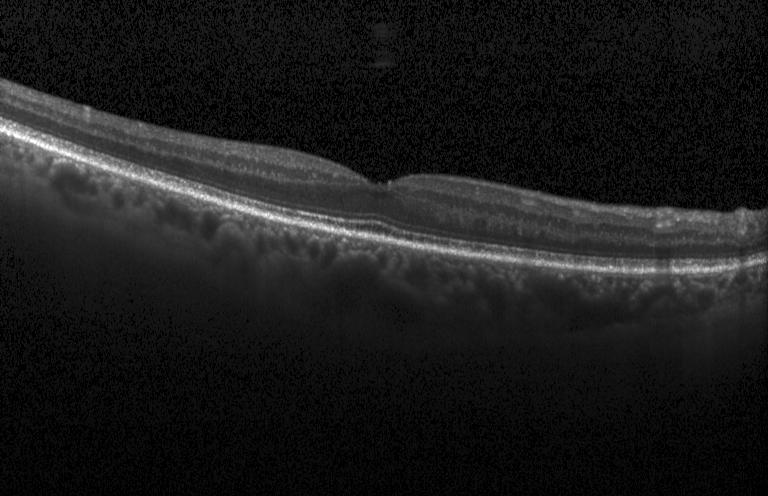 Finding: neither choroidal neovascularization, diabetic macular edema, nor drusen.